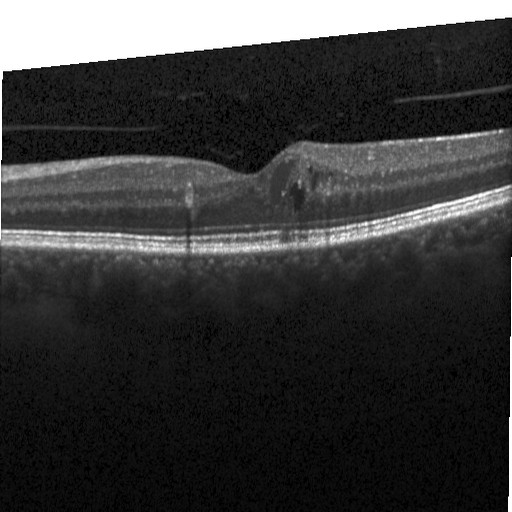 Optical coherence tomography B-scan, centered on the fovea
Macular OCT: diabetic macular edema (DME).